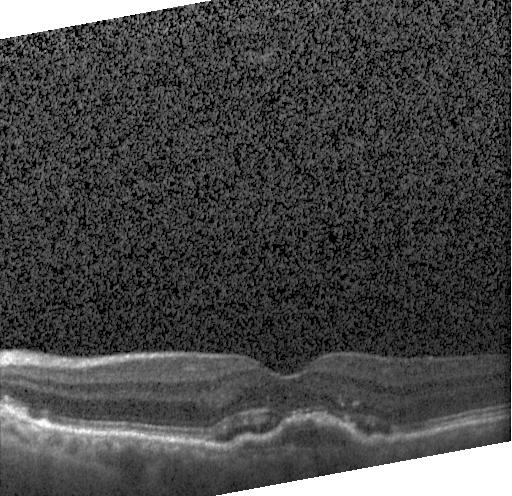

OCT scan showing CNV.